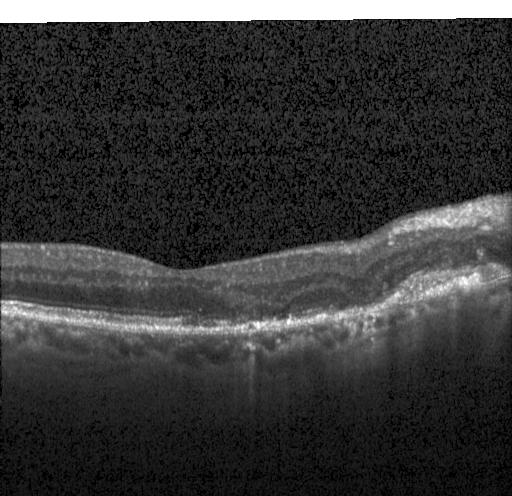
Retinal OCT cross-section, macular scan, spectral-domain OCT, acquired on a Heidelberg Spectralis. Choroidal neovascularization.